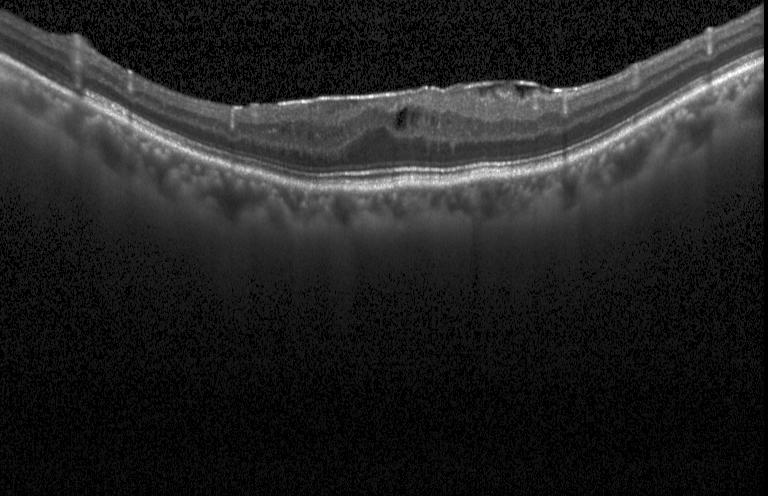 OCT B-scan · fovea-centered · Heidelberg Spectralis OCT system · spectral-domain optical coherence tomography
Macular OCT: DME.